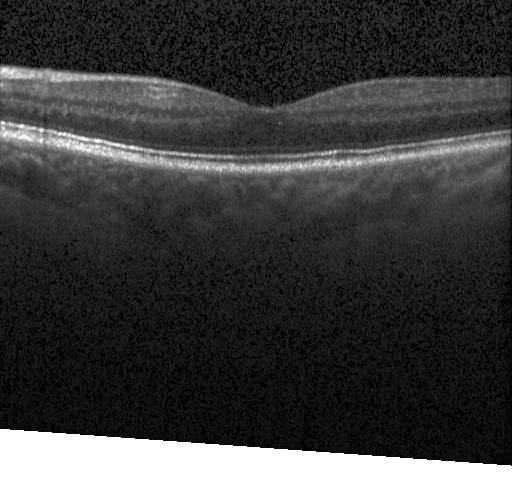
Finding: no CNV, no DME, and no drusen.